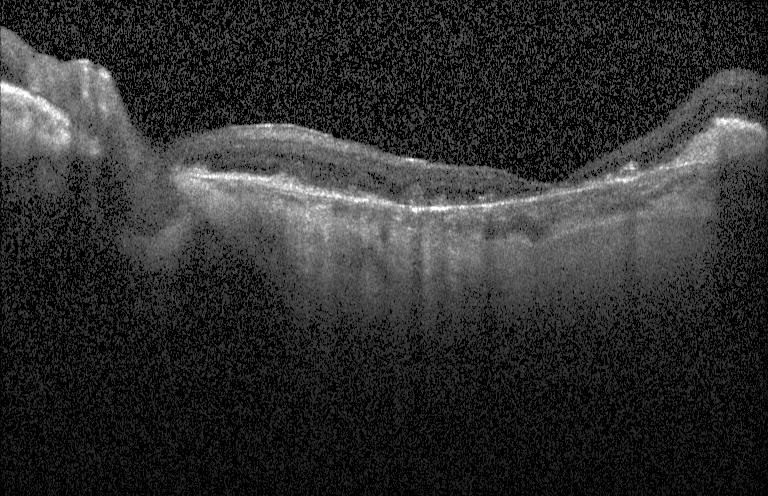 Retinal OCT cross-section showing choroidal neovascularization (CNV).